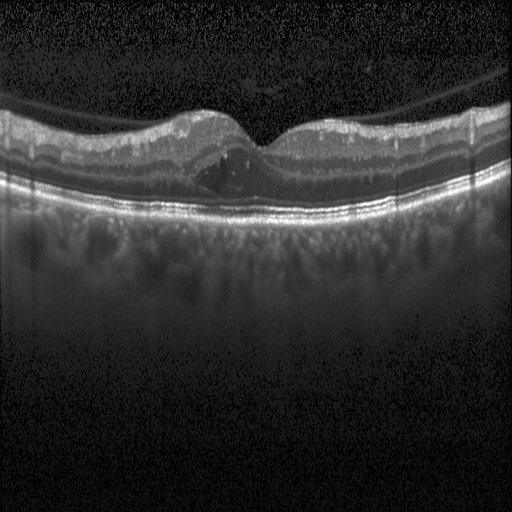

Spectral-domain optical coherence tomography. Through the macula. Instrument: Heidelberg Spectralis. OCT B-scan. The scan shows diabetic macular edema.